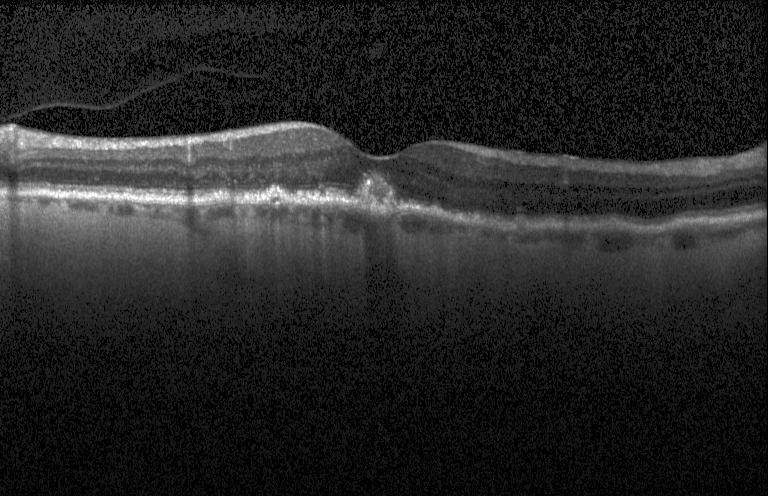 OCT B-scan; through the macula; spectral-domain optical coherence tomography; acquired on a Heidelberg Spectralis.
The scan shows sub-RPE drusenoid deposits.